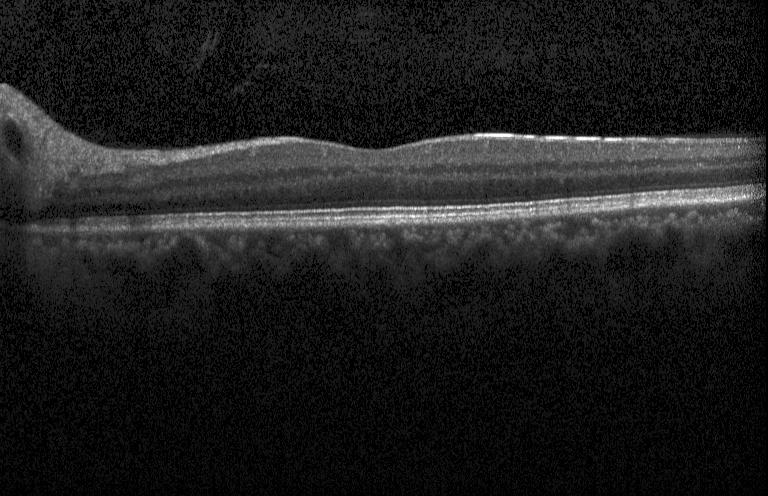 OCT B-scan, SD-OCT, acquired on a Heidelberg Spectralis, horizontal scan through the fovea
Finding: no evidence of choroidal neovascularization, diabetic macular edema, or drusen.